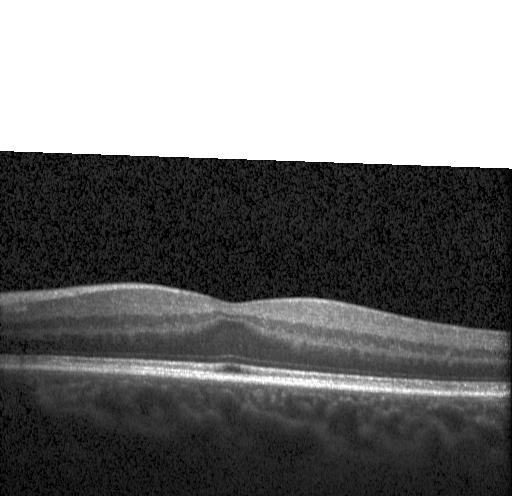 Spectral-domain optical coherence tomography. Retinal OCT cross-section — Macular OCT: no choroidal neovascularization, diabetic macular edema, or drusen.